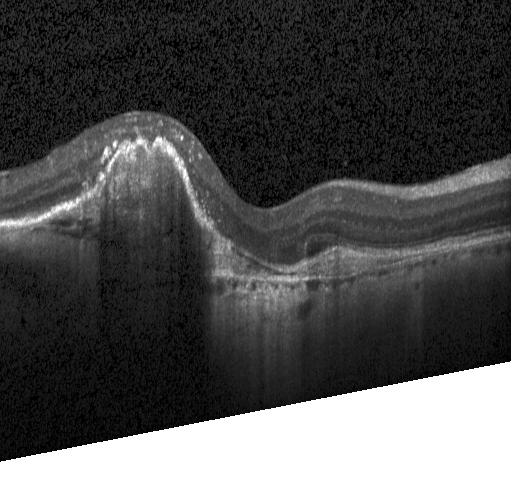 Retinal OCT cross-section
Finding: CNV.